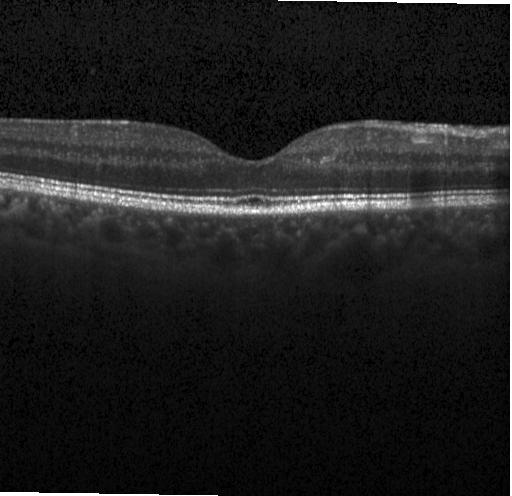 Finding: no choroidal neovascularization, no diabetic macular edema, and no drusen.